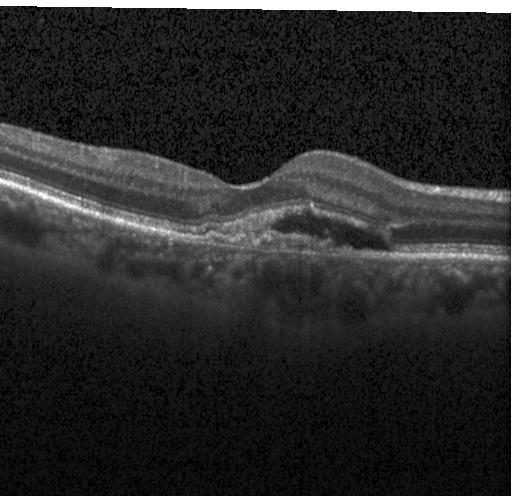

Horizontal scan through the fovea · OCT B-scan — OCT finding: a choroidal neovascular membrane.